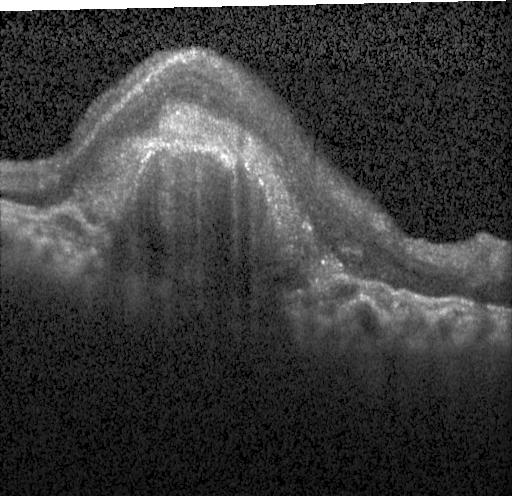 Retinal OCT cross-section; fovea-centered; Heidelberg Spectralis OCT system. Assessment: choroidal neovascularization.